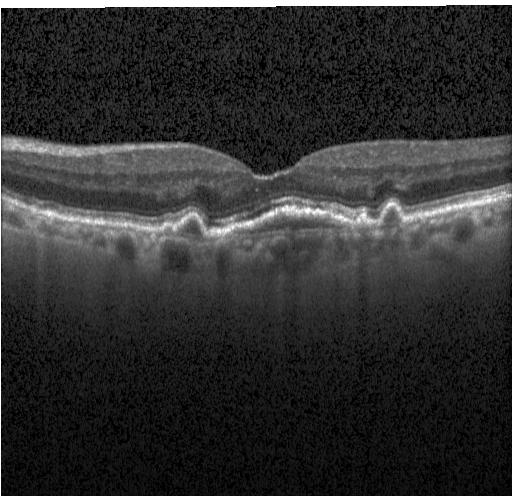

OCT line scan. OCT finding: a choroidal neovascular membrane.